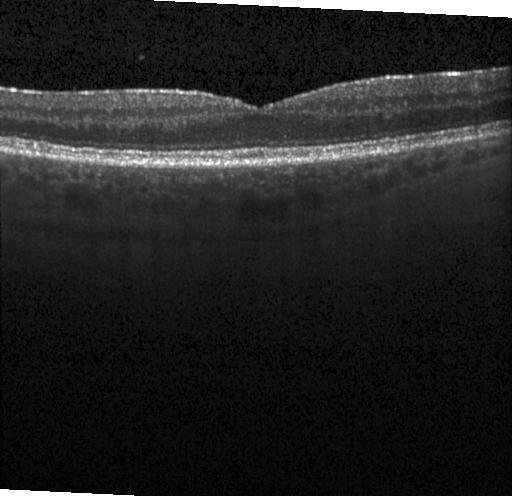
Optical coherence tomography B-scan · spectral-domain optical coherence tomography
Finding: neither choroidal neovascularization, diabetic macular edema, nor drusen.